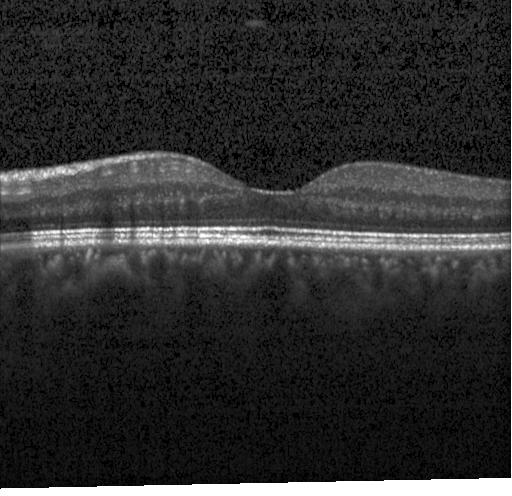 Macular scan, spectral-domain OCT, retinal OCT cross-section. Assessment: no evidence of CNV, DME, or drusen.